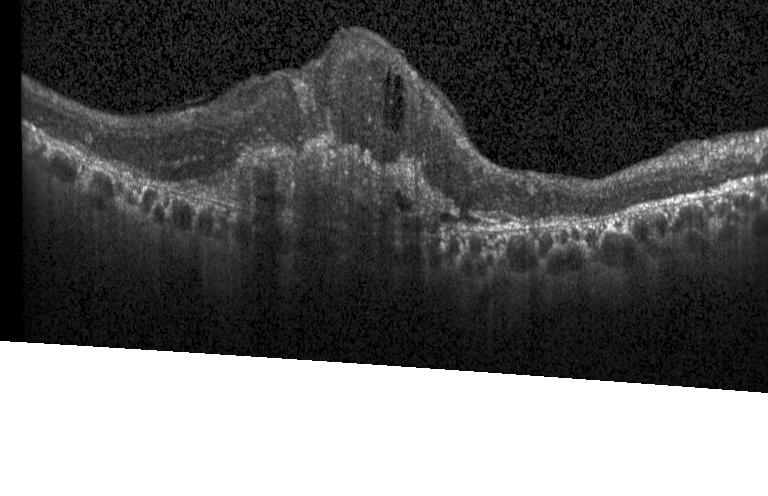 Impression: a choroidal neovascular membrane.